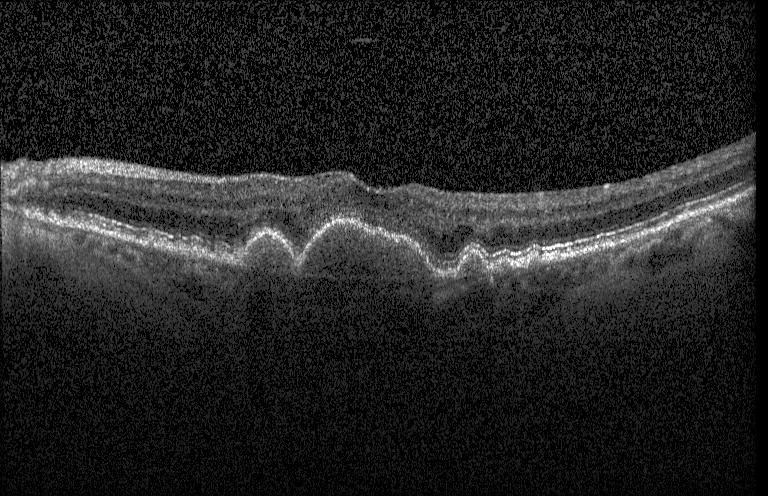

Retinal OCT B-scan
Impression: a choroidal neovascular membrane.